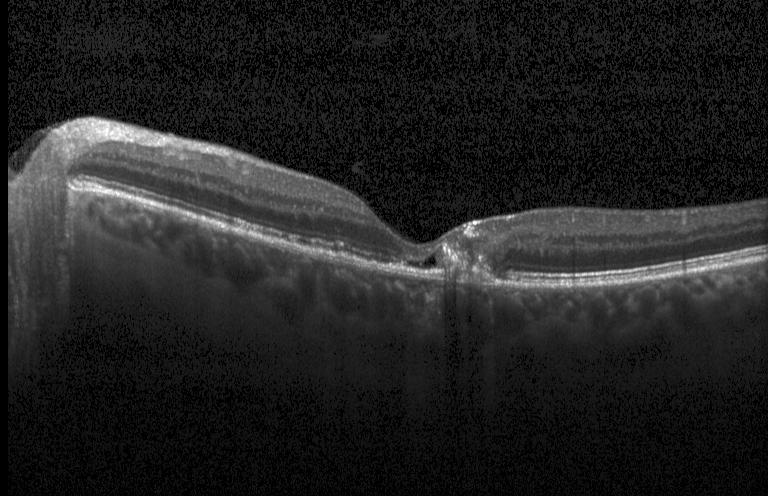

Heidelberg Spectralis OCT system · macular scan · optical coherence tomography B-scan
A choroidal neovascular membrane.